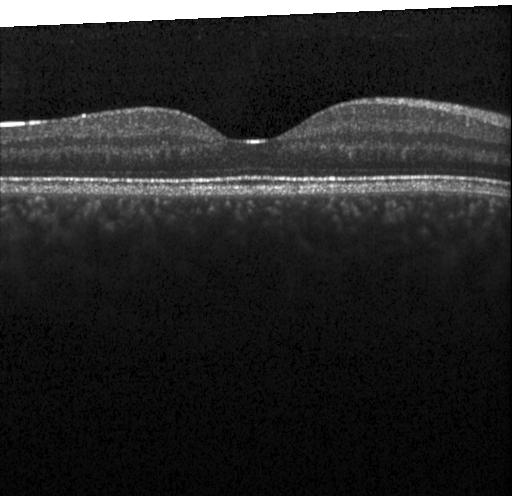
Impression: no CNV, no DME, and no drusen.